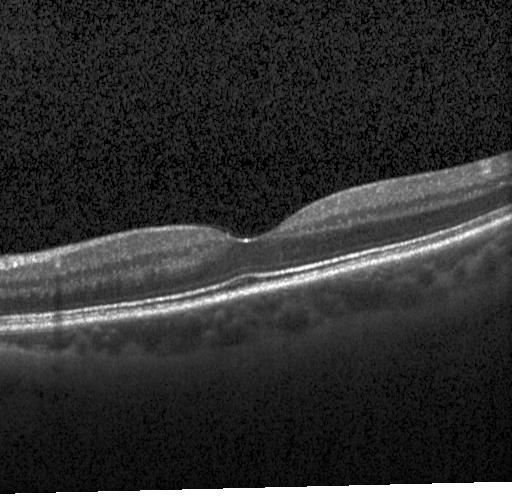
Heidelberg Spectralis · retinal OCT B-scan · horizontal scan through the fovea. The scan shows no choroidal neovascularization, no diabetic macular edema, and no drusen.